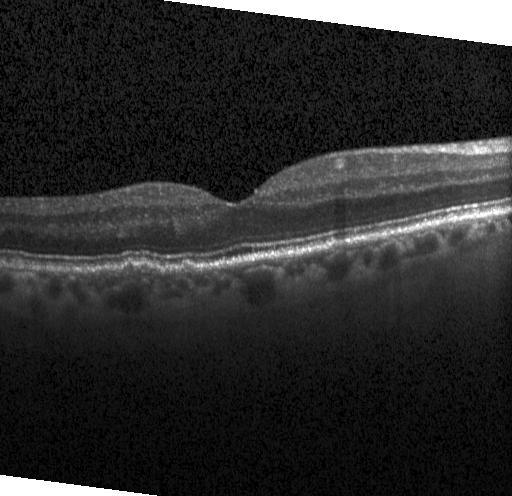

Finding: sub-RPE drusenoid deposits.